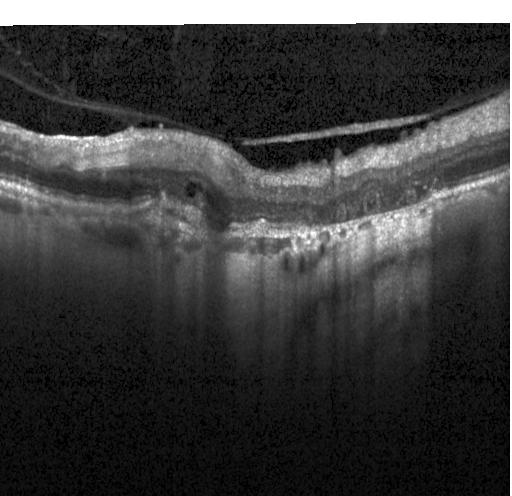
Heidelberg Spectralis OCT system, centered on the fovea, retinal OCT B-scan. Assessment: a choroidal neovascular membrane.